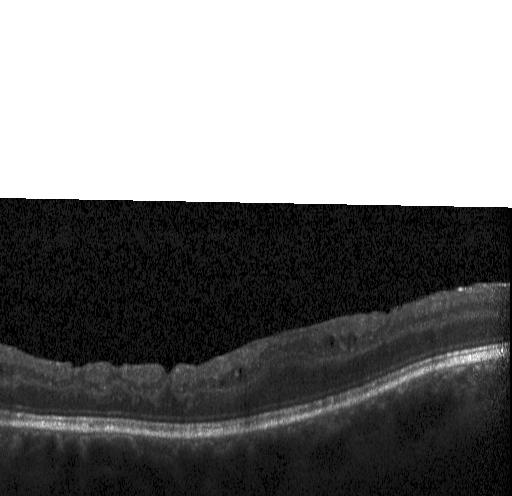

Through the macula, OCT line scan.
Dx: diabetic macular edema.